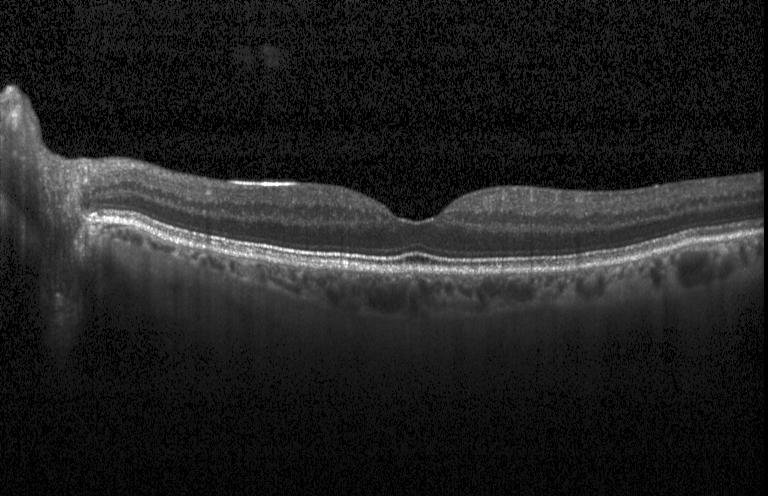

Spectral-domain optical coherence tomography. OCT line scan. Macular scan. Finding: no evidence of CNV, DME, or drusen.